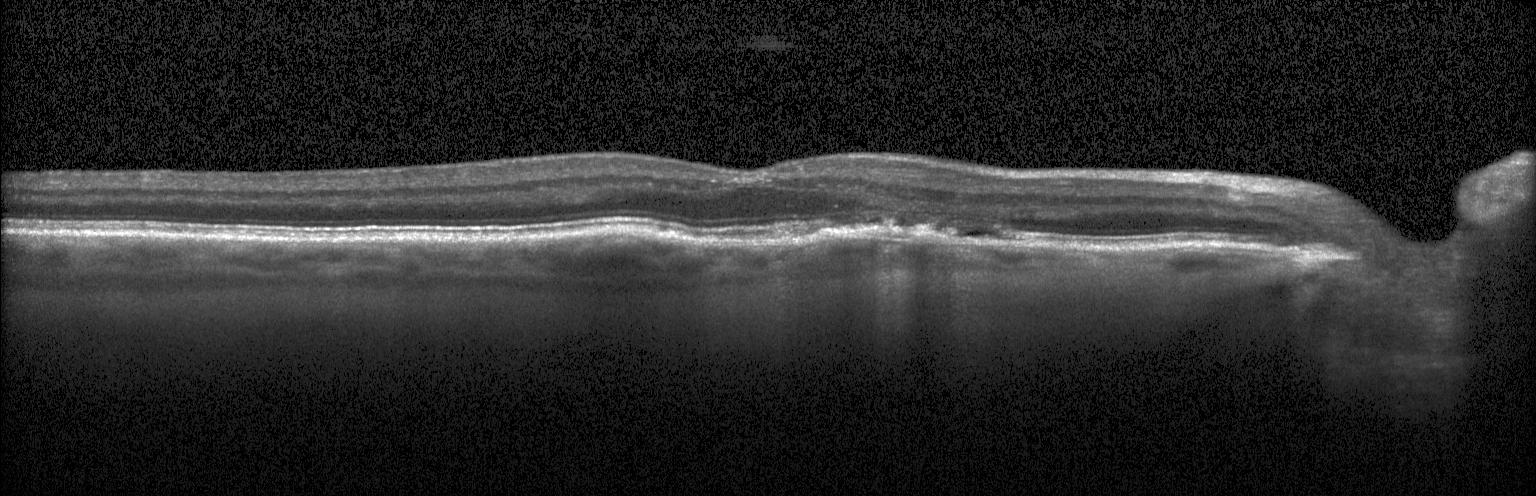 Macular scan, SD-OCT, OCT line scan, instrument: Heidelberg Spectralis
This B-scan demonstrates CNV.